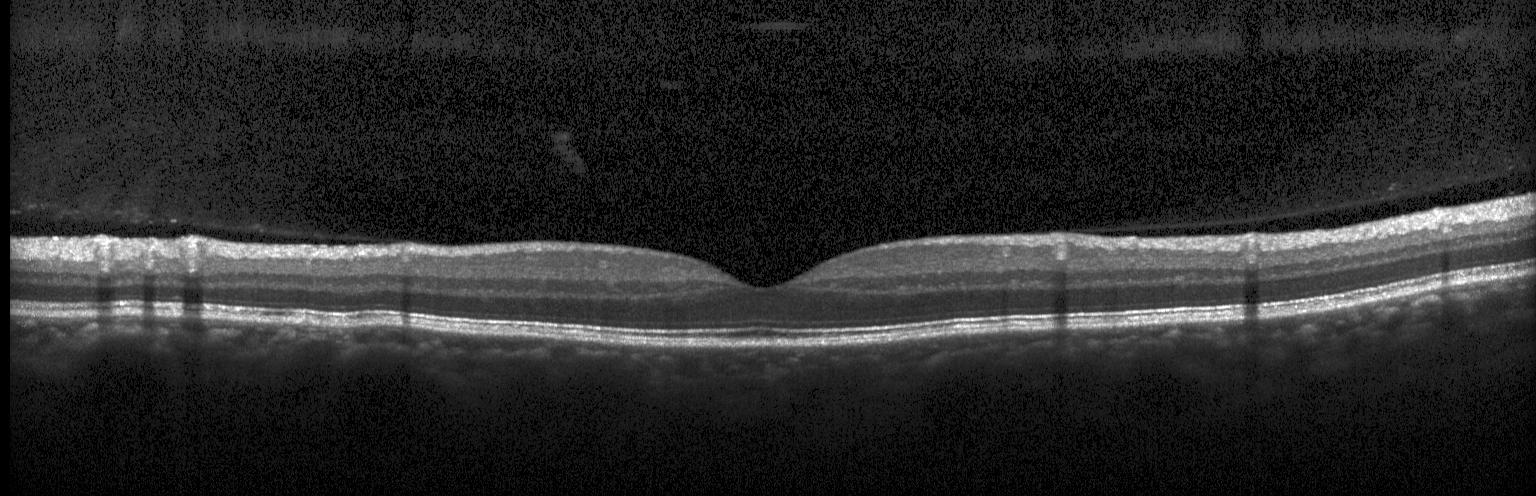

OCT B-scan.
Finding: neither choroidal neovascularization, diabetic macular edema, nor drusen.